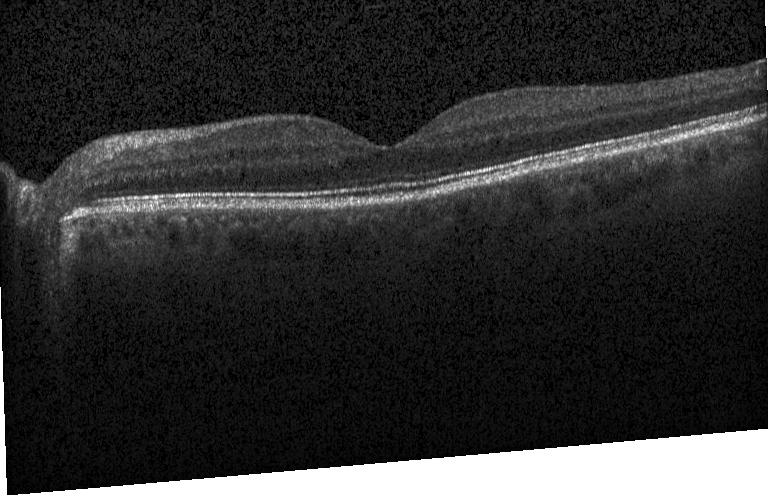

Spectral-domain OCT B-scan: no CNV, no DME, and no drusen.